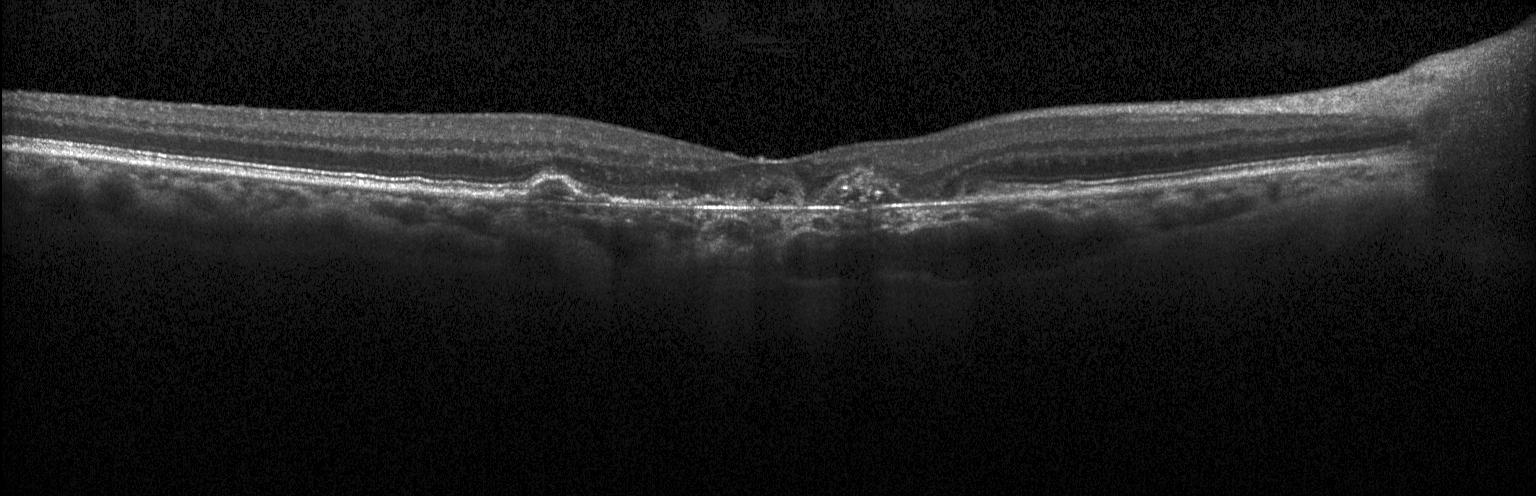
Finding: choroidal neovascularization.